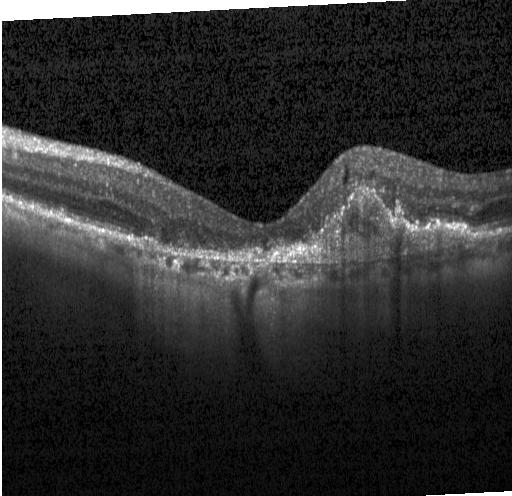

OCT line scan, through the macula — This B-scan demonstrates a choroidal neovascular membrane.